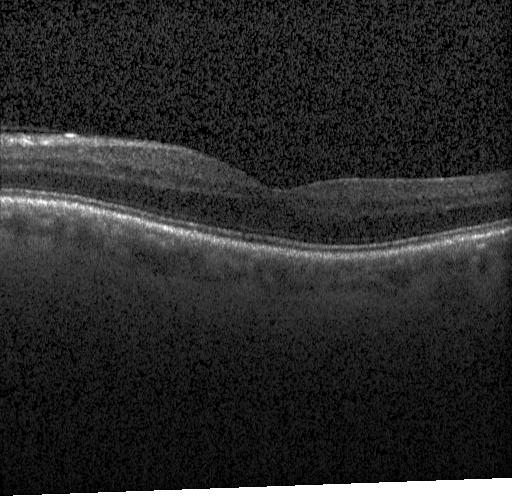
Heidelberg Spectralis · optical coherence tomography scan · macular scan. No choroidal neovascularization, no diabetic macular edema, and no drusen.